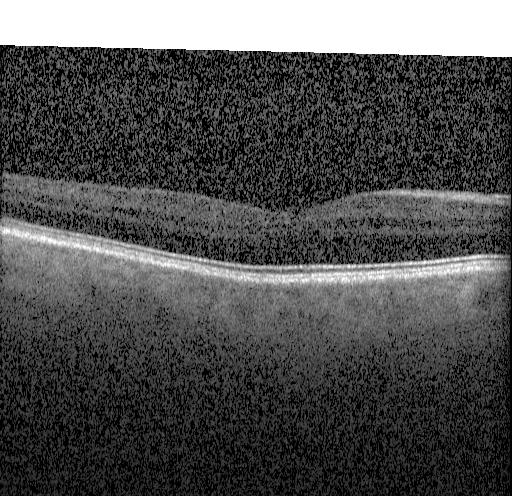
Impression: no CNV, no DME, and no drusen.